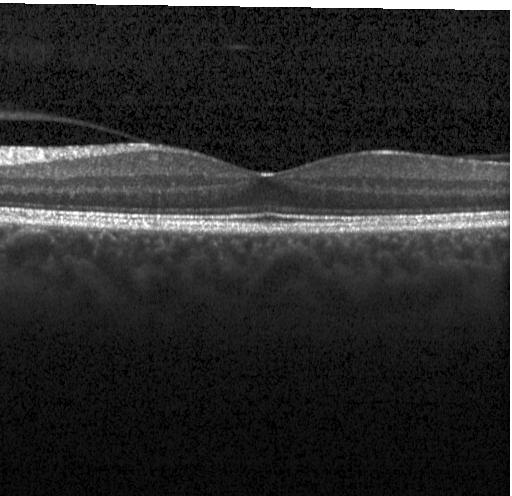 Instrument: Heidelberg Spectralis · spectral-domain optical coherence tomography · OCT B-scan — Diagnosis: no CNV, no DME, and no drusen.